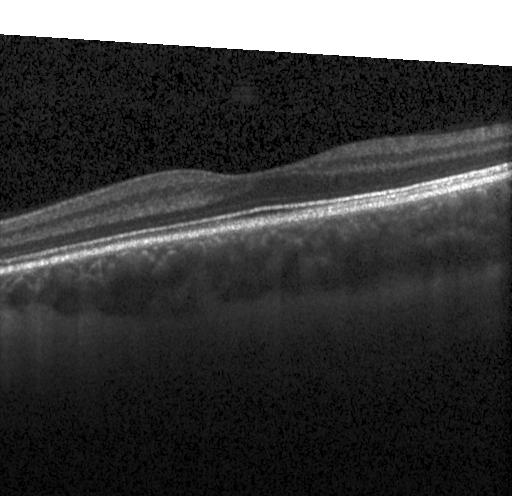

Instrument: Heidelberg Spectralis. Macular scan. SD-OCT. Retinal OCT cross-section — Neither choroidal neovascularization, diabetic macular edema, nor drusen.